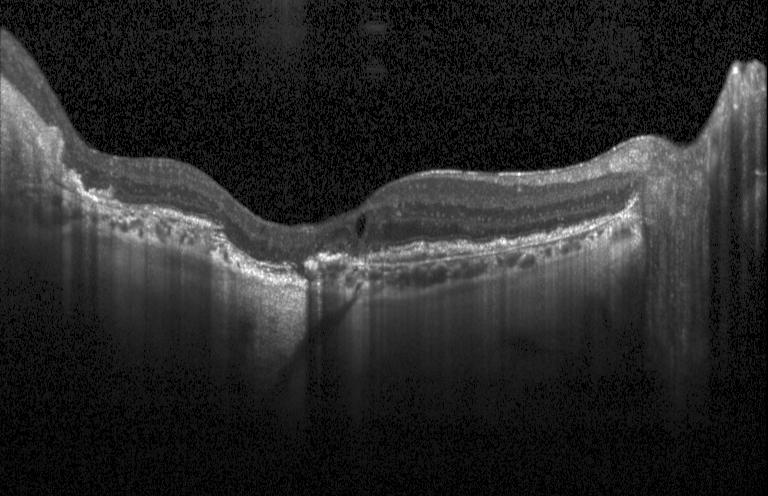
Dx: CNV.